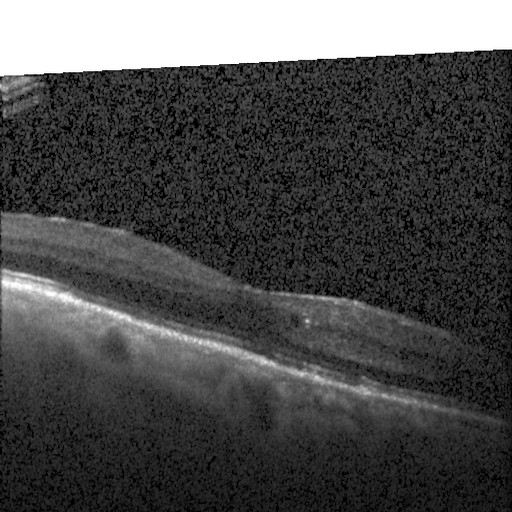 SD-OCT; OCT line scan; acquired on a Heidelberg Spectralis; macular scan — This B-scan demonstrates diabetic macular edema.